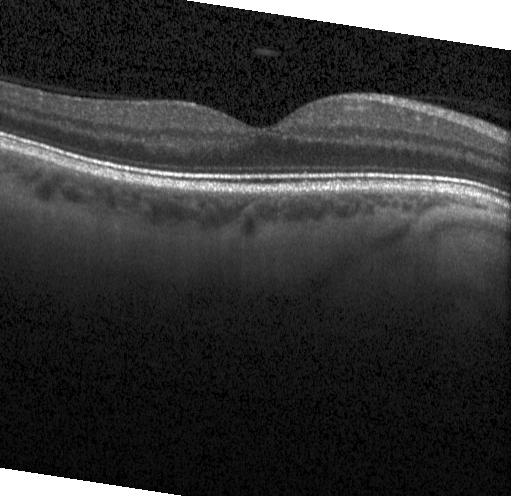
Macular OCT: no choroidal neovascularization, no diabetic macular edema, and no drusen.